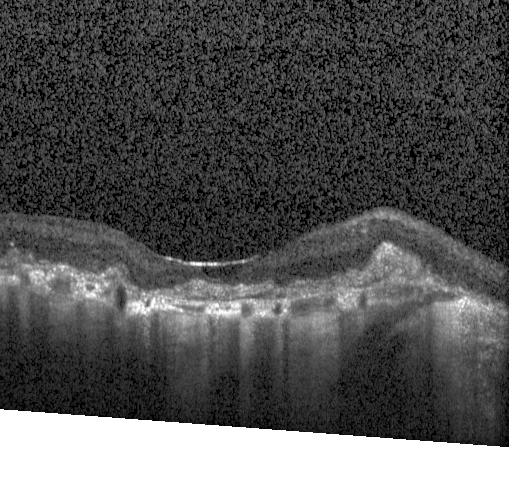 Diagnosis: choroidal neovascularization (CNV).